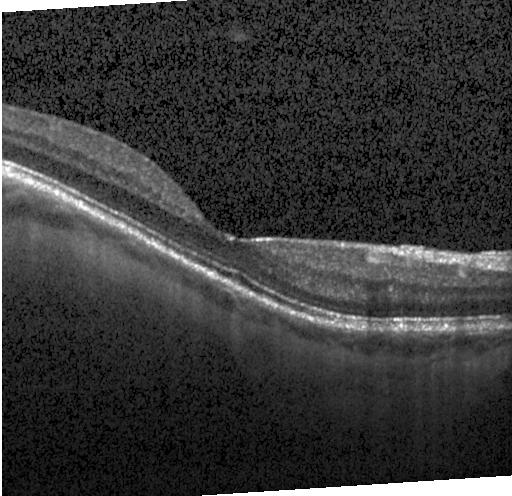

OCT B-scan showing no evidence of choroidal neovascularization, diabetic macular edema, or drusen.